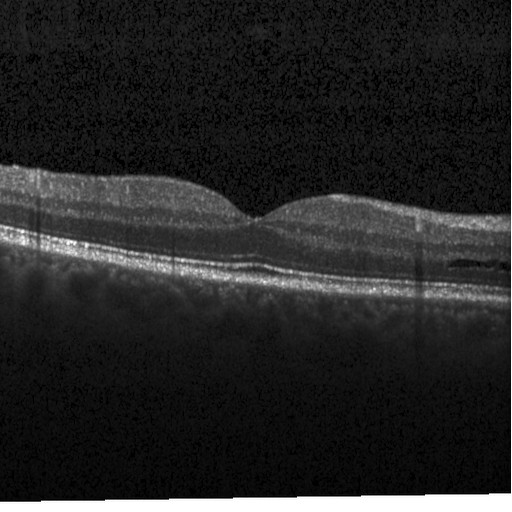

This B-scan demonstrates DME.